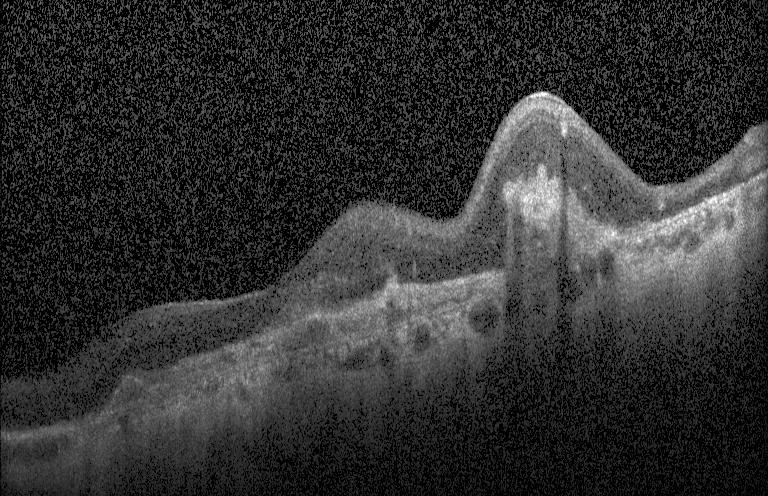
Macular OCT demonstrating a choroidal neovascular membrane.